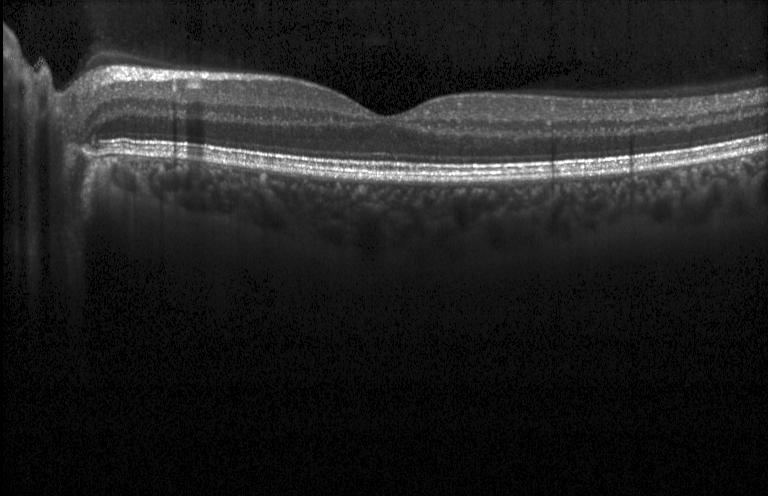
Spectral-domain OCT B-scan: no choroidal neovascularization, diabetic macular edema, or drusen.